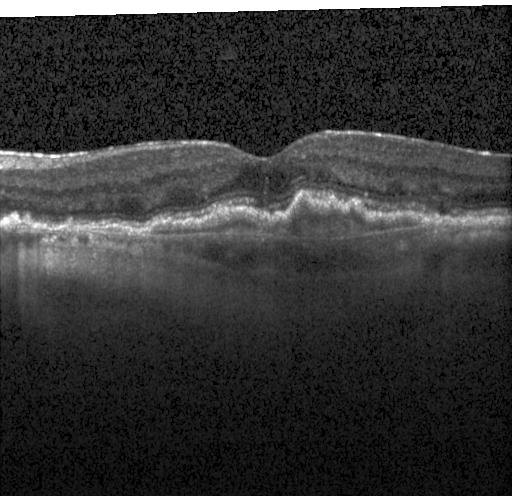

Retinal OCT cross-section.
Diagnosis: a choroidal neovascular membrane.